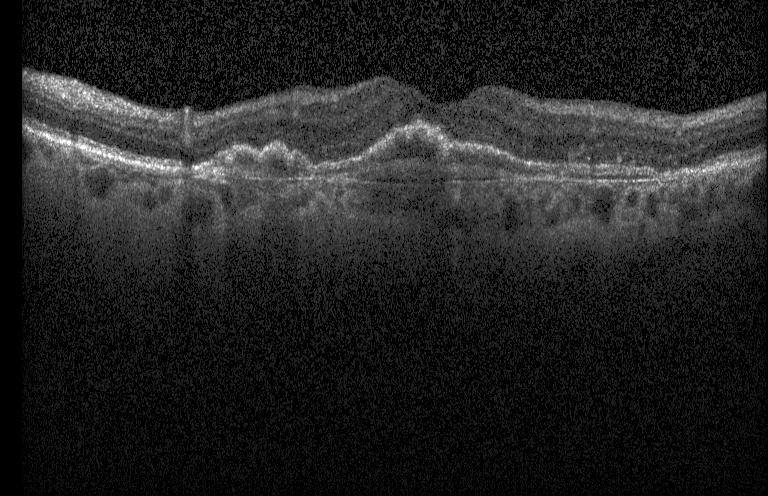 Heidelberg Spectralis; retinal OCT B-scan
Finding: a choroidal neovascular membrane.